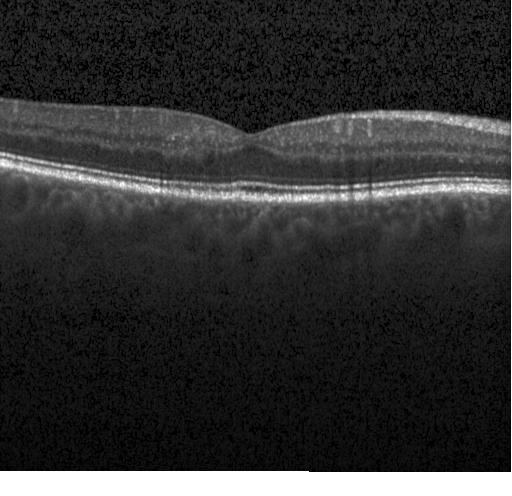 Macular OCT: no evidence of choroidal neovascularization, diabetic macular edema, or drusen.